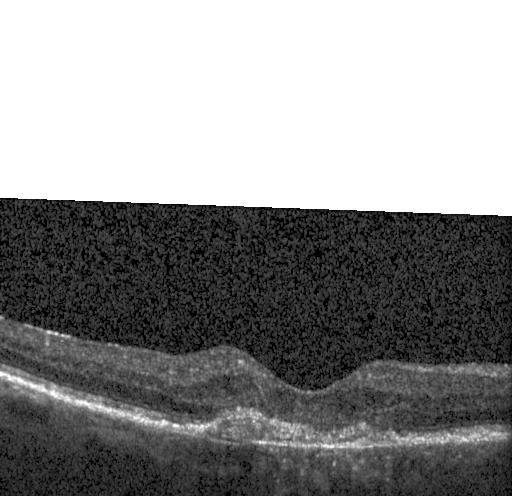 OCT scan showing a choroidal neovascular membrane.